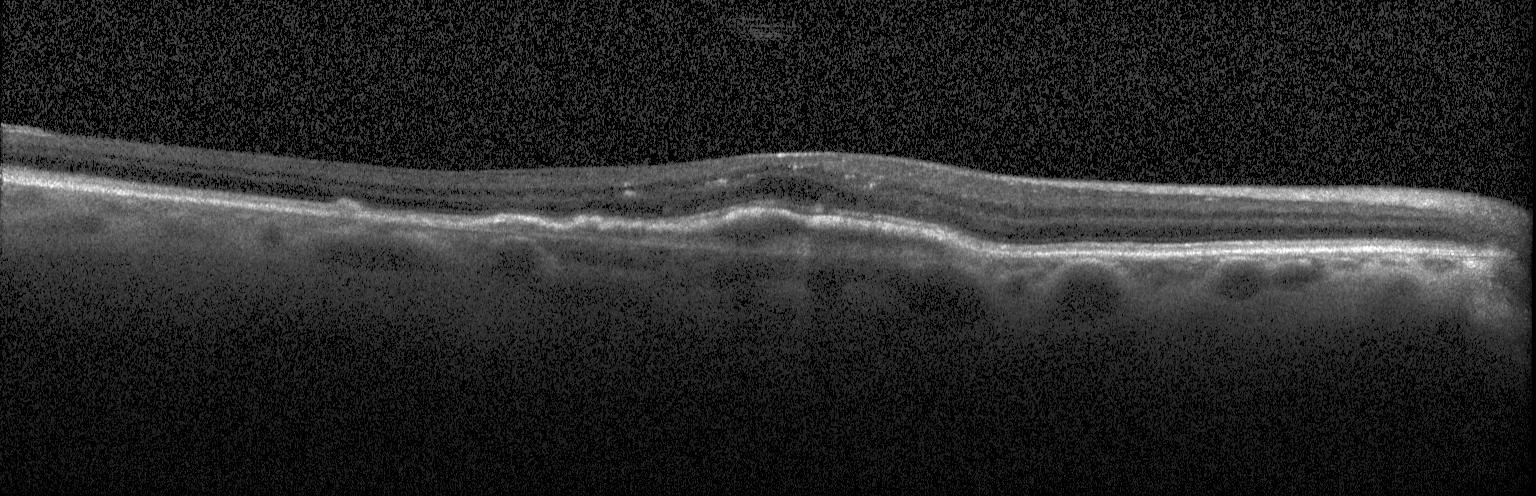
OCT B-scan.
Assessment: a choroidal neovascular membrane.